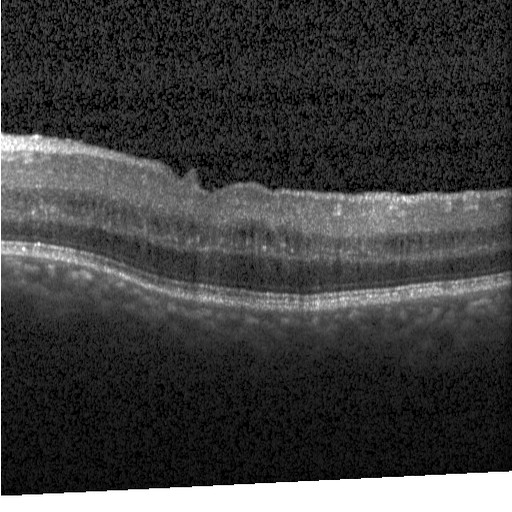
Finding: diabetic macular edema.